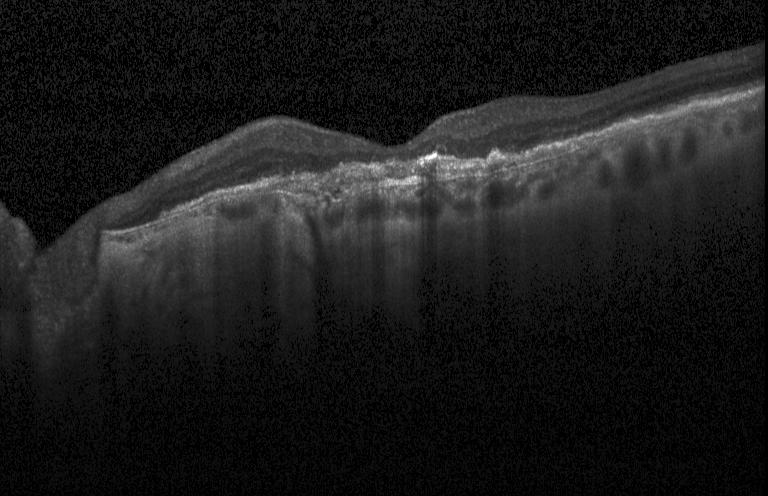 Retinal OCT cross-section.
Diagnosis: a choroidal neovascular membrane.